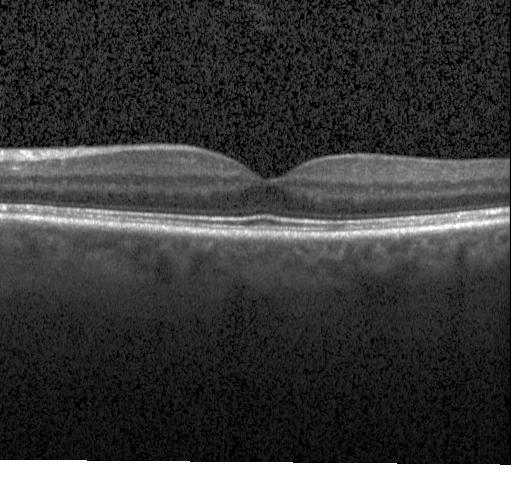
OCT B-scan — Finding: neither CNV, DME, nor drusen.